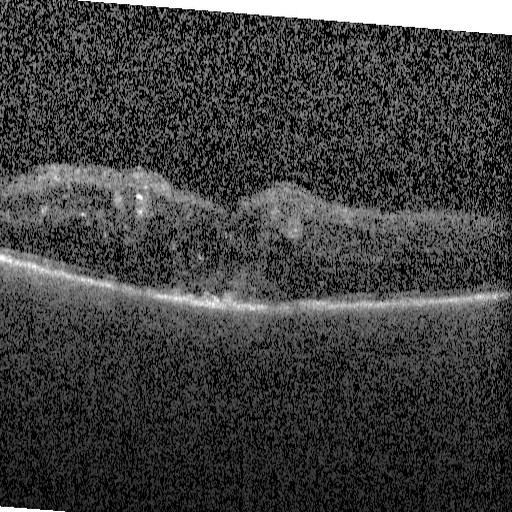 Impression: DME.